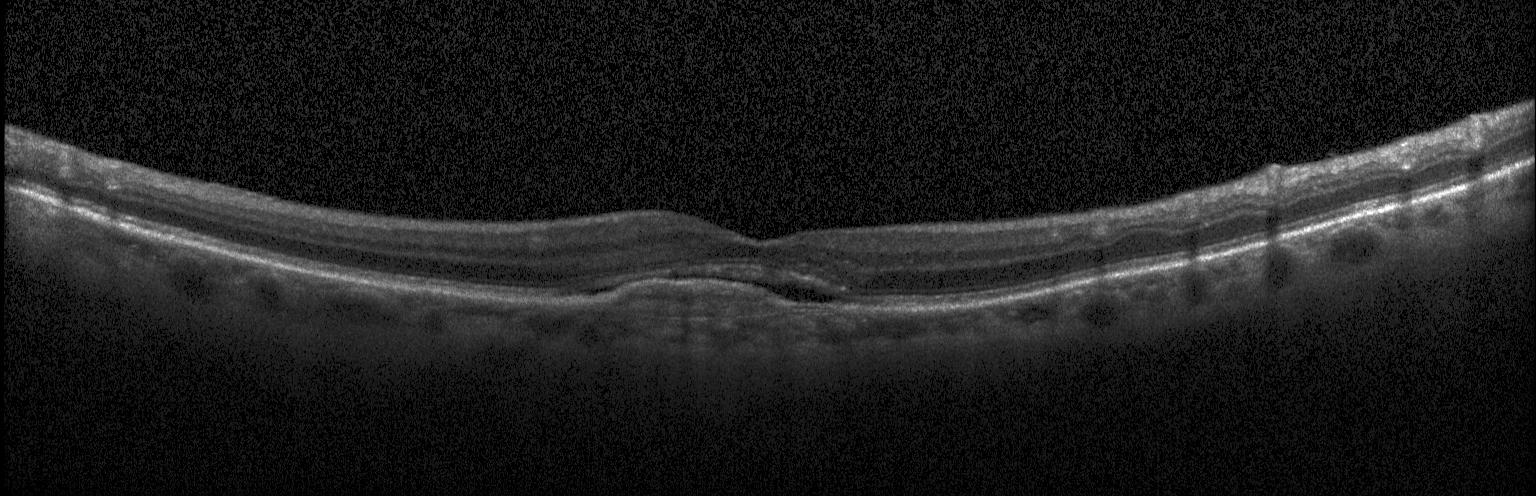

Acquired on a Heidelberg Spectralis. Optical coherence tomography B-scan.
Impression: choroidal neovascularization.